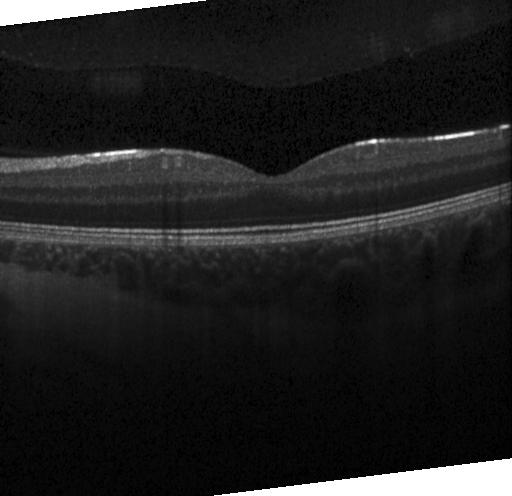
Spectral-domain OCT; retinal OCT cross-section
OCT finding: neither CNV, DME, nor drusen.